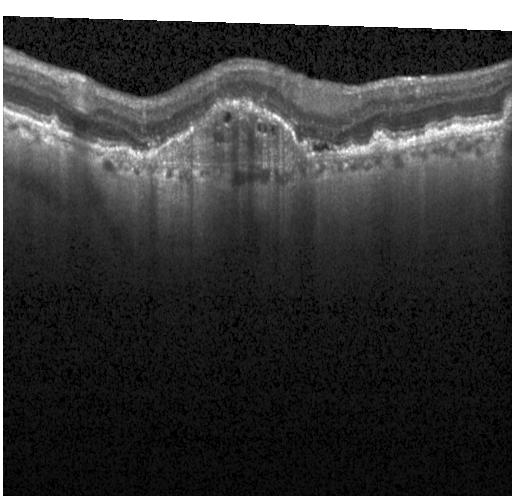 OCT line scan.
The scan shows choroidal neovascularization.